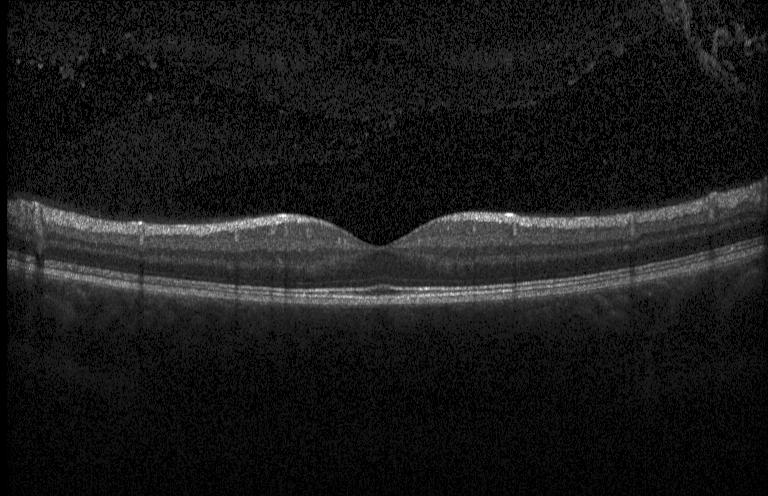 Spectral-domain optical coherence tomography. Through the macula. Optical coherence tomography B-scan — Impression: no CNV, no DME, and no drusen.